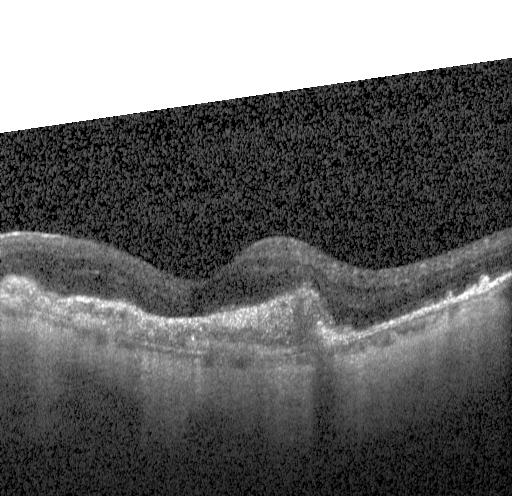

OCT line scan. Fovea-centered.
Diagnosis: CNV.